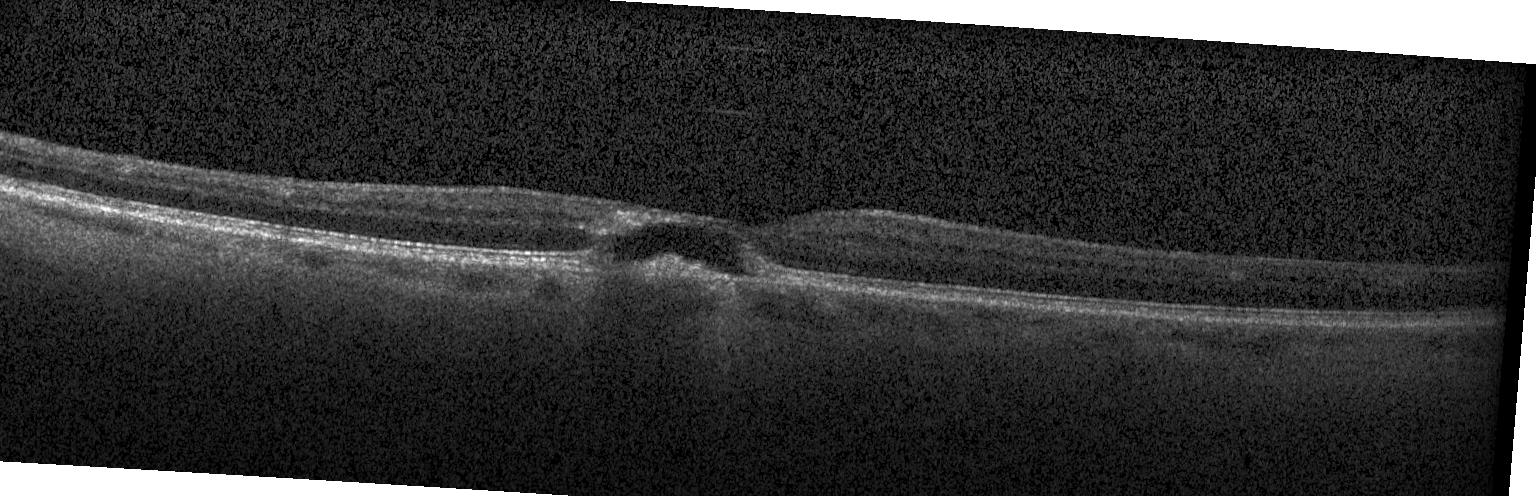 Acquired on a Heidelberg Spectralis. Retinal OCT cross-section. Spectral-domain optical coherence tomography.
Impression: choroidal neovascularization (CNV).